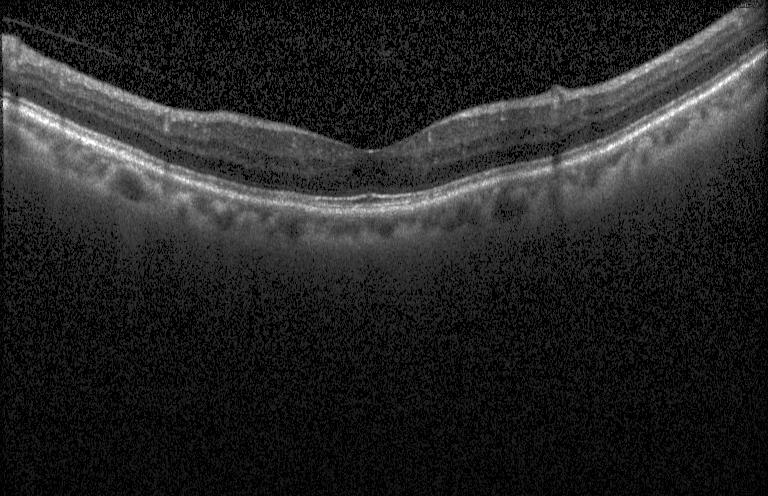
Spectral-domain optical coherence tomography; retinal OCT B-scan. Assessment: no choroidal neovascularization, diabetic macular edema, or drusen.